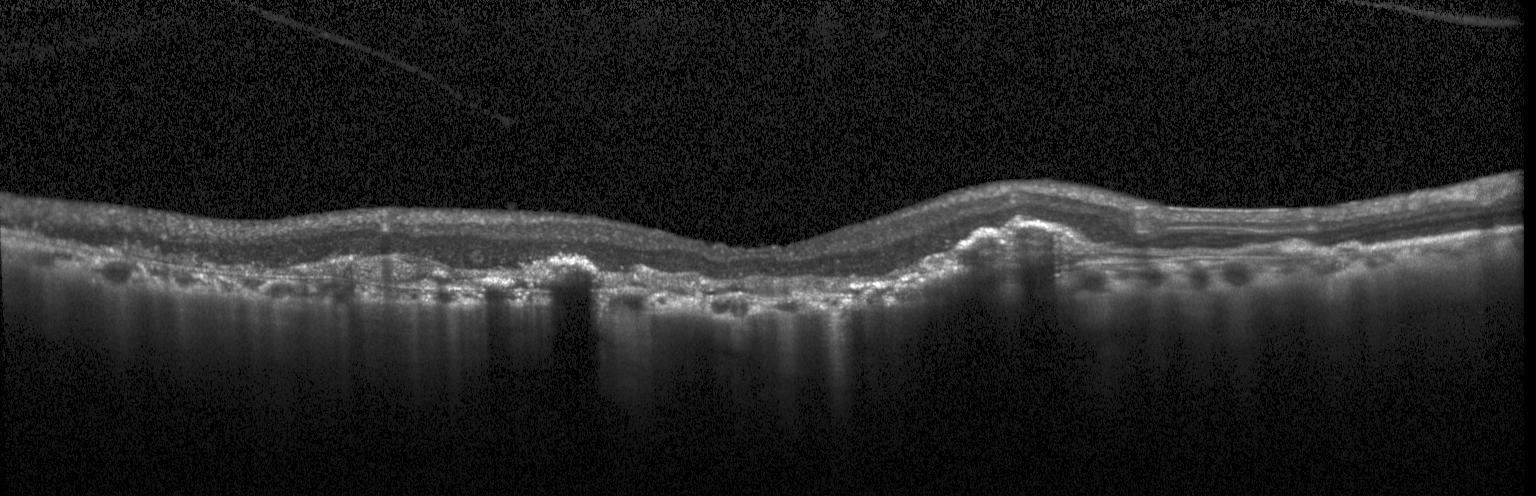
The scan shows choroidal neovascularization.